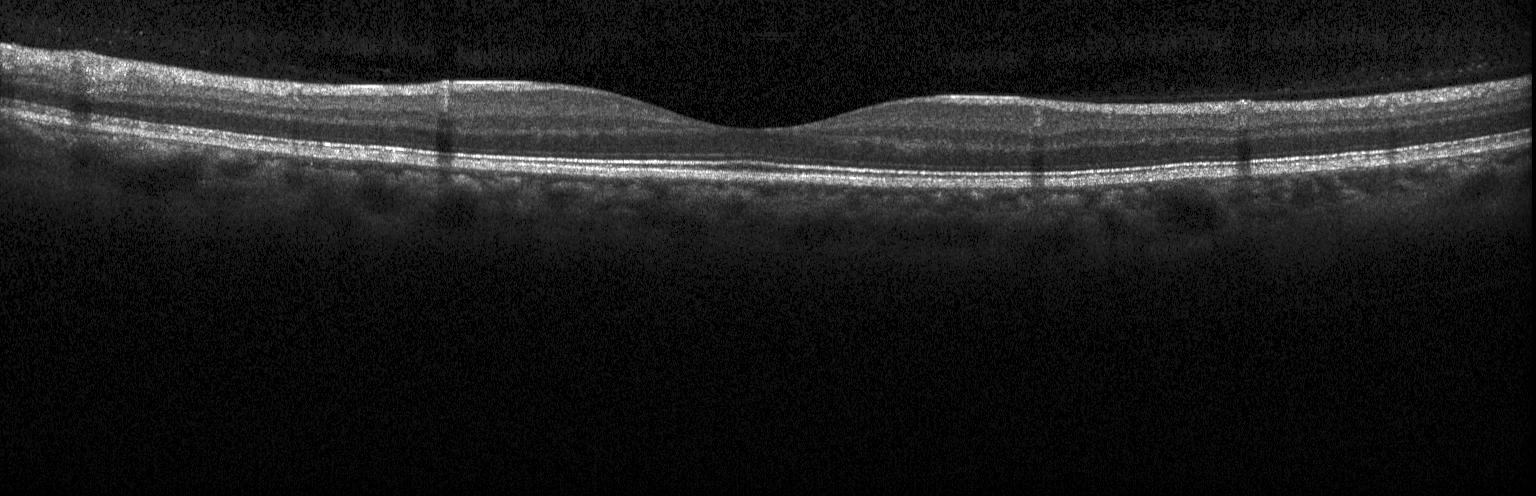
Centered on the fovea. Instrument: Heidelberg Spectralis. Optical coherence tomography B-scan. SD-OCT. This B-scan demonstrates no CNV, DME, or drusen.